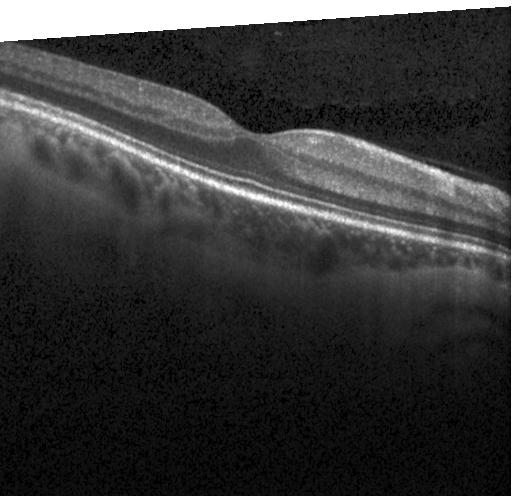

Retinal OCT B-scan.
Impression: no evidence of choroidal neovascularization, diabetic macular edema, or drusen.